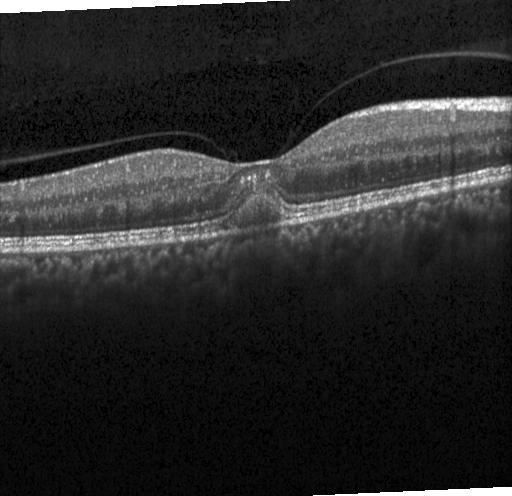
Retinal OCT B-scan. The scan shows a choroidal neovascular membrane.